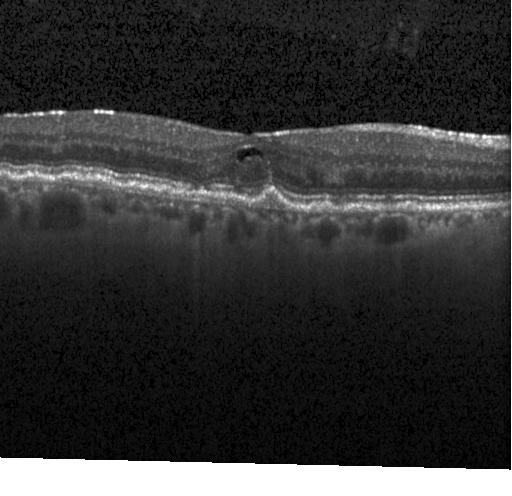 Retinal OCT B-scan; spectral-domain optical coherence tomography
Choroidal neovascularization (CNV).